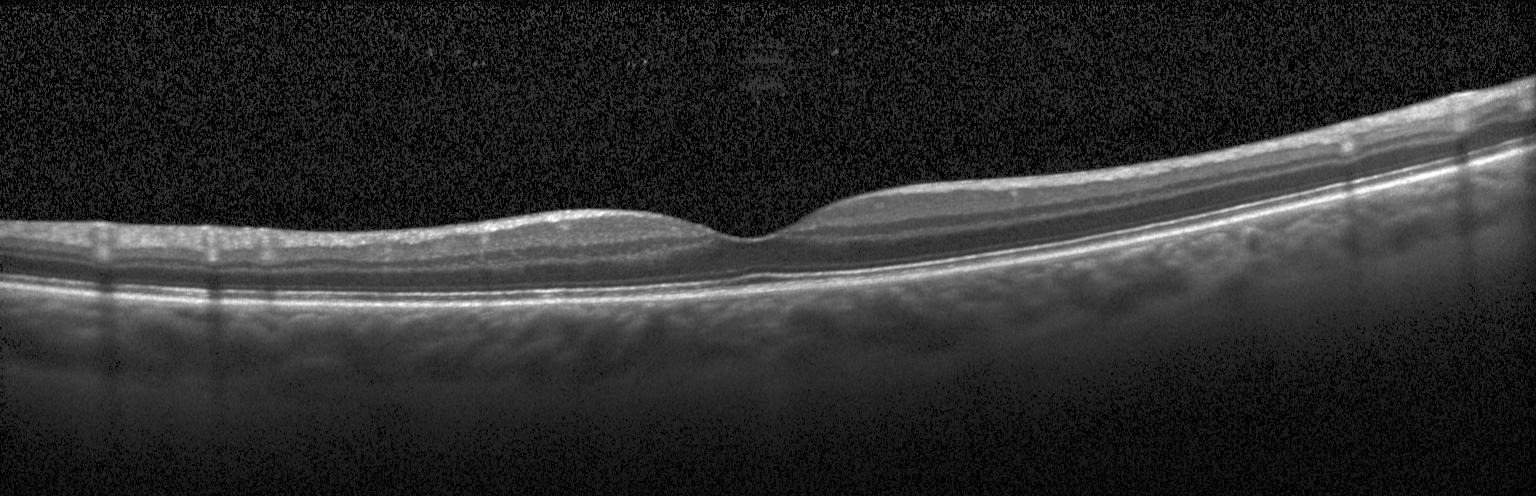
This B-scan demonstrates no choroidal neovascularization, diabetic macular edema, or drusen.